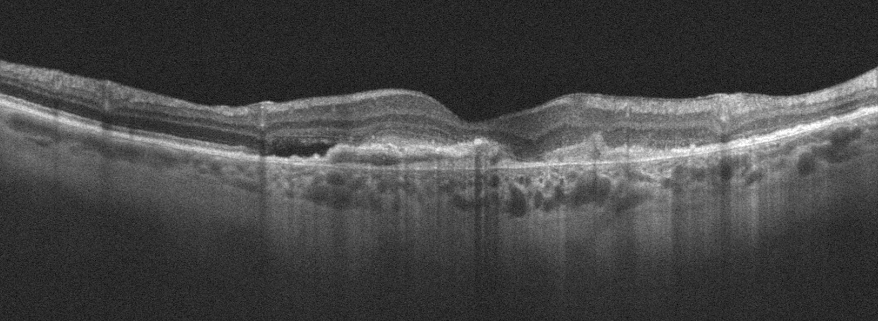 Retinal OCT B-scan.
Impression: age-related macular degeneration.